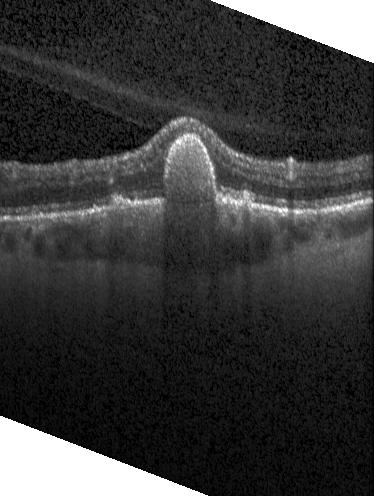

Through the macula. Heidelberg Spectralis OCT system. Optical coherence tomography scan. Impression: CNV.